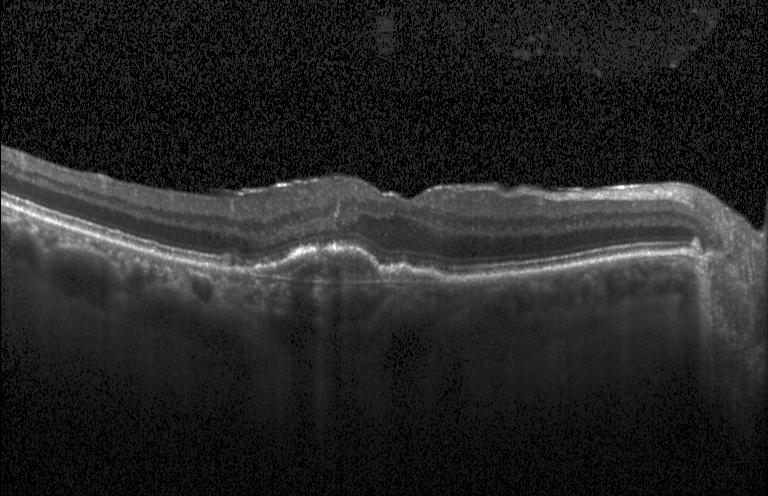

Optical coherence tomography B-scan.
Finding: a choroidal neovascular membrane.